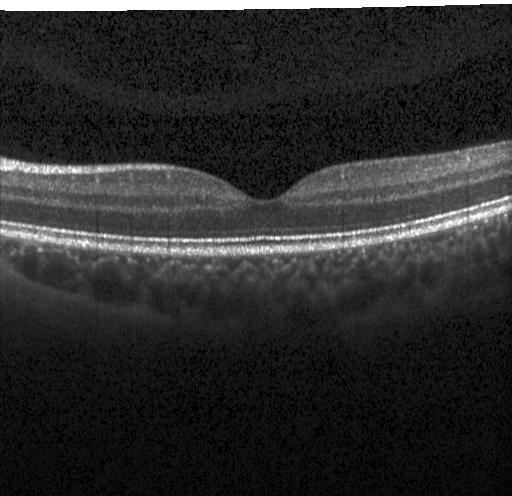
OCT B-scan. Assessment: neither choroidal neovascularization, diabetic macular edema, nor drusen.